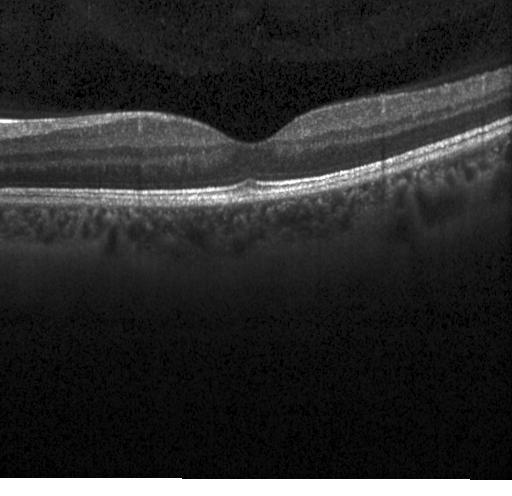

Heidelberg Spectralis OCT system. Optical coherence tomography scan. Spectral-domain optical coherence tomography. Horizontal scan through the fovea
Diagnosis: no evidence of CNV, DME, or drusen.